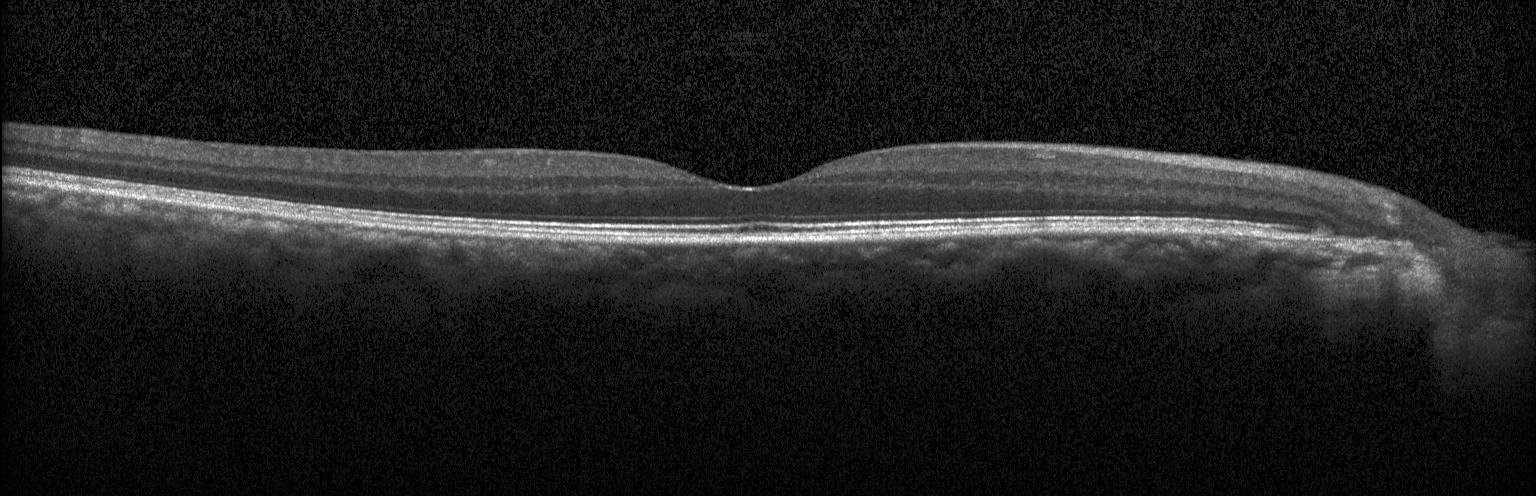
The scan shows neither CNV, DME, nor drusen.